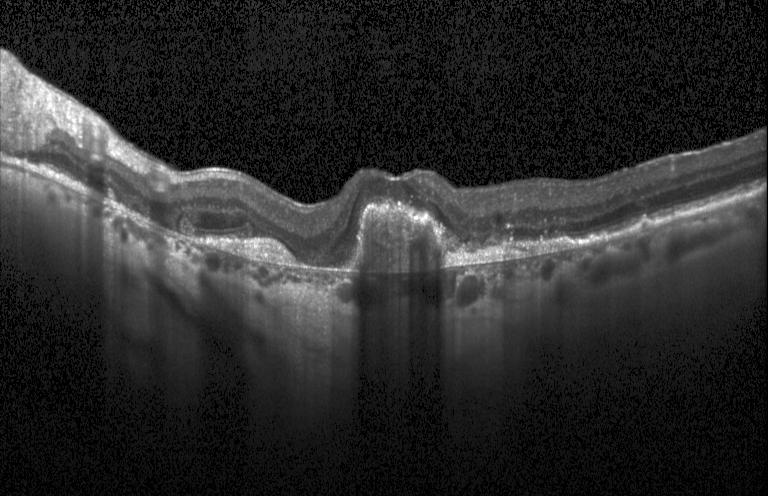
OCT B-scan showing choroidal neovascularization (CNV).